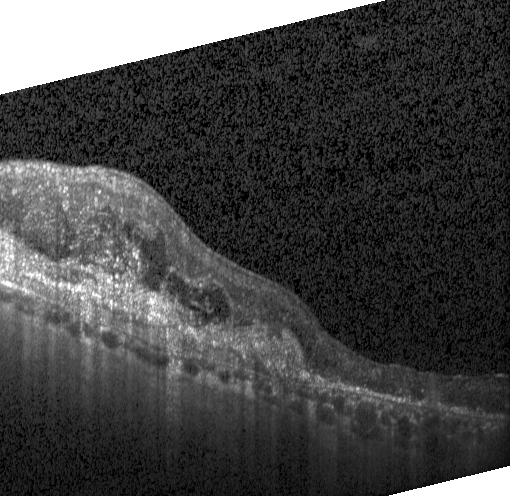
Macular OCT: a choroidal neovascular membrane.